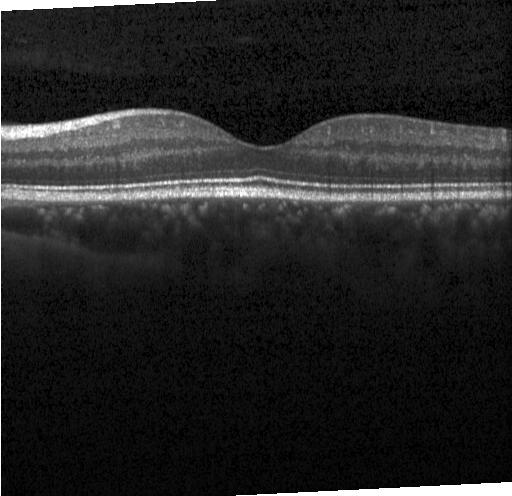
Diagnosis: no evidence of choroidal neovascularization, diabetic macular edema, or drusen.